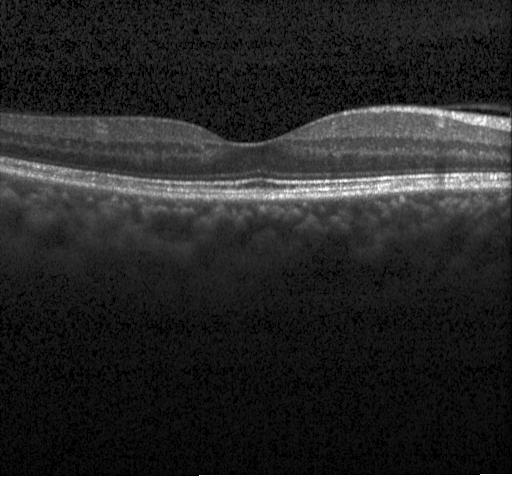

Spectral-domain OCT B-scan: neither CNV, DME, nor drusen.